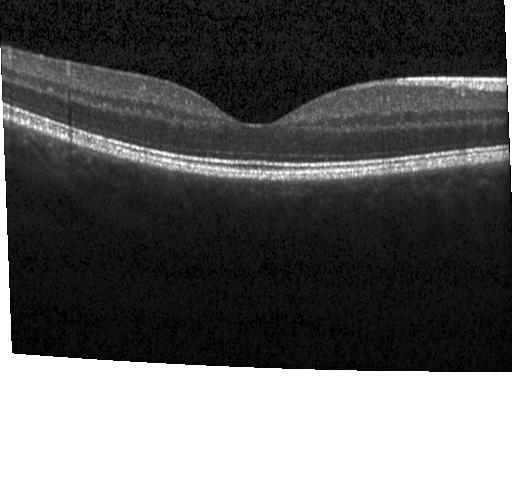 OCT line scan · instrument: Heidelberg Spectralis · spectral-domain OCT.
Diagnosis: no choroidal neovascularization, no diabetic macular edema, and no drusen.